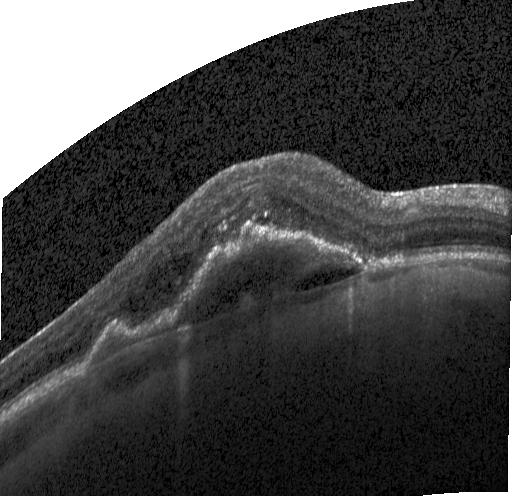
Macular scan; Heidelberg Spectralis OCT system; spectral-domain OCT; retinal OCT B-scan.
Macular OCT: CNV.